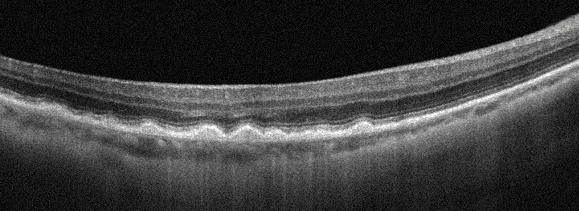
Right eye. Retinal OCT B-scan — Impression: AMD.